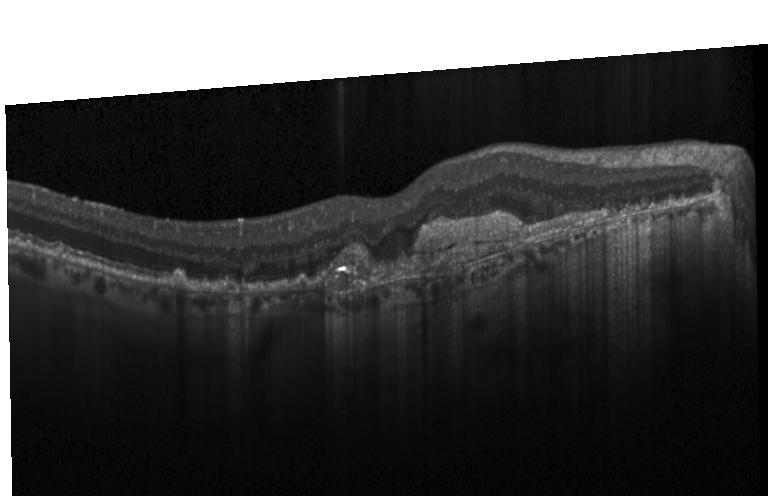 Retinal OCT B-scan. Finding: a choroidal neovascular membrane.